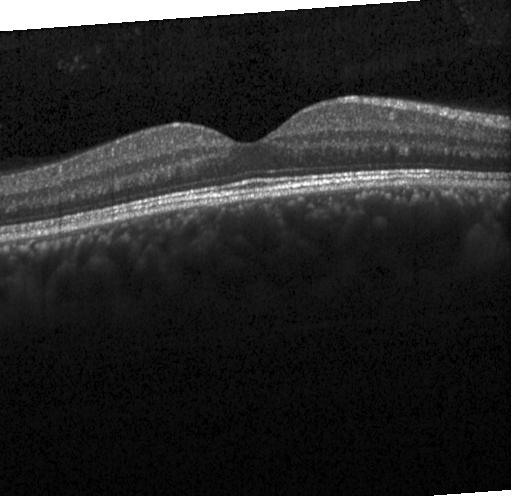 Optical coherence tomography scan · through the macula · SD-OCT — This B-scan demonstrates no evidence of choroidal neovascularization, diabetic macular edema, or drusen.